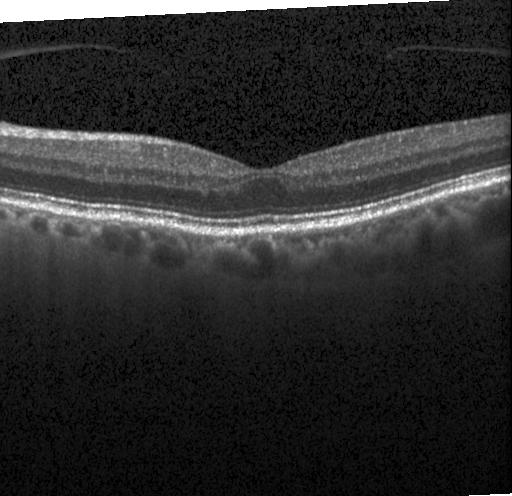 OCT B-scan showing no CNV, DME, or drusen.